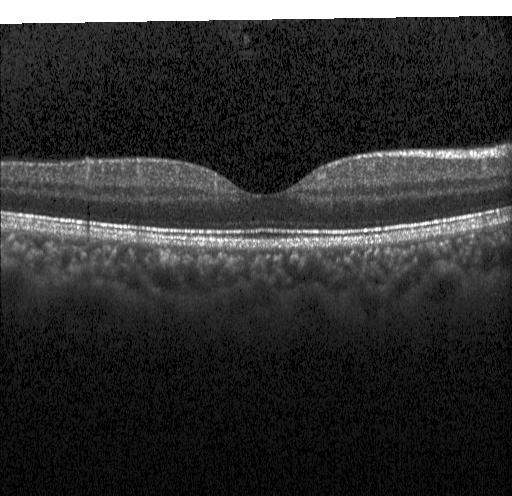

Optical coherence tomography B-scan · spectral-domain OCT — Dx: no evidence of CNV, DME, or drusen.